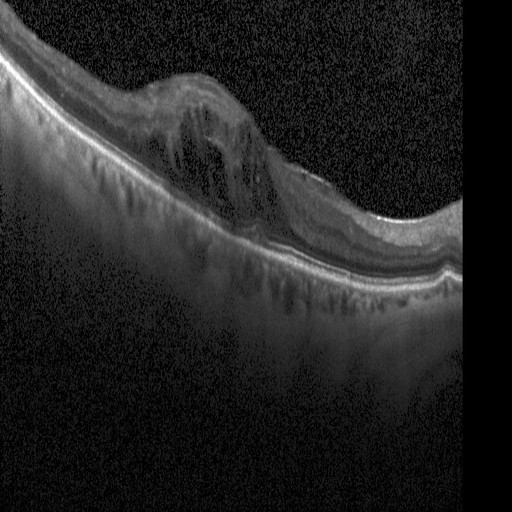

Spectral-domain optical coherence tomography, optical coherence tomography scan — This B-scan demonstrates diabetic macular edema.